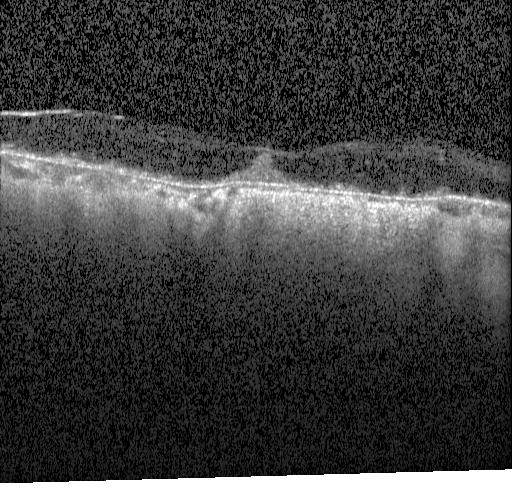 Instrument: Heidelberg Spectralis. Spectral-domain optical coherence tomography. Retinal OCT cross-section
The scan shows a choroidal neovascular membrane.